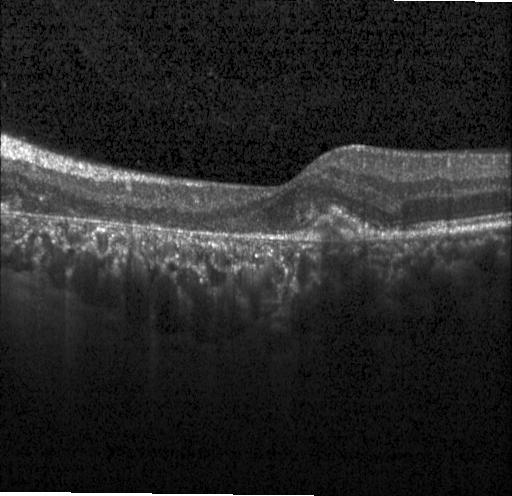
Retinal OCT B-scan
Dx: CNV.